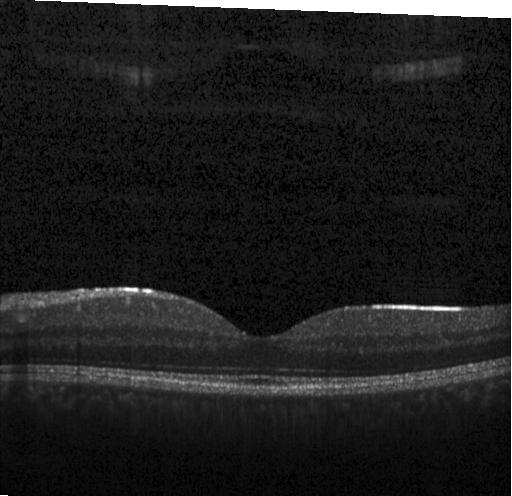
Retinal OCT cross-section; spectral-domain OCT; instrument: Heidelberg Spectralis; through the macula.
The scan shows no choroidal neovascularization, diabetic macular edema, or drusen.